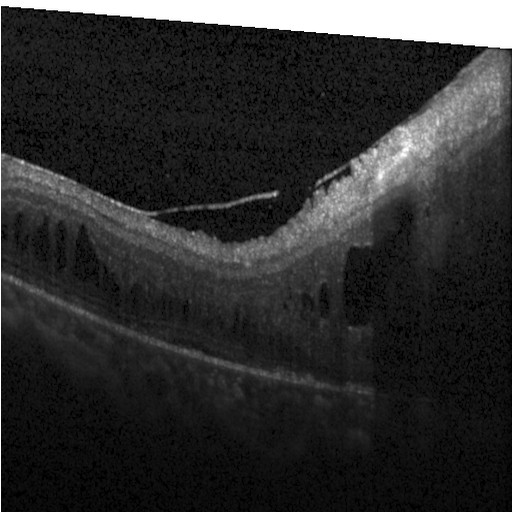 Fovea-centered, Heidelberg Spectralis, optical coherence tomography scan, spectral-domain OCT — Macular OCT: diabetic macular edema.